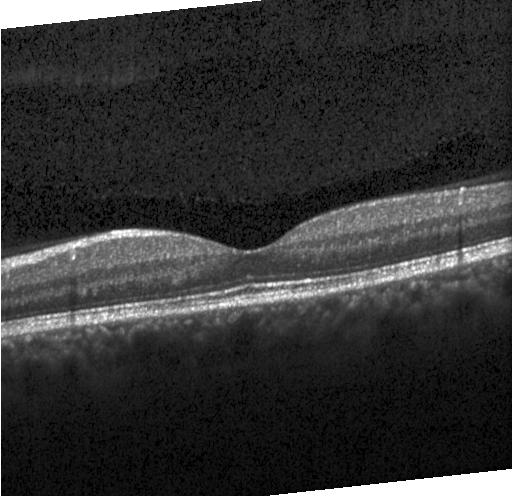 Optical coherence tomography scan; SD-OCT; through the macula. Impression: no choroidal neovascularization, no diabetic macular edema, and no drusen.